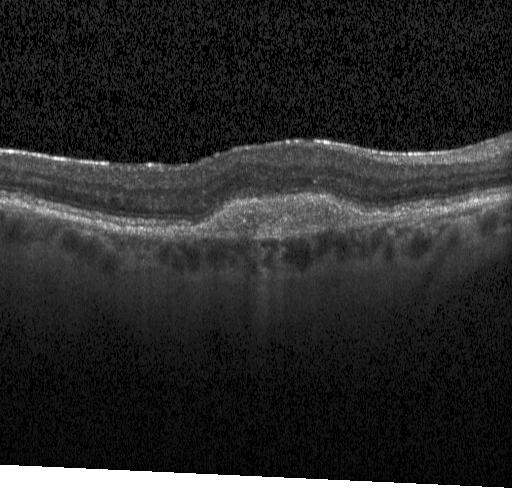
Spectral-domain OCT B-scan: a choroidal neovascular membrane.